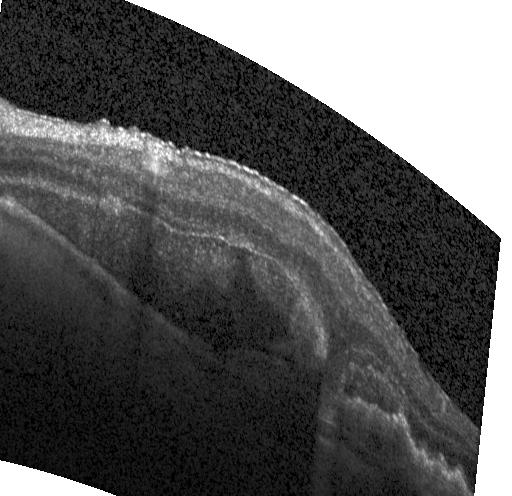
Retinal OCT cross-section showing a choroidal neovascular membrane.